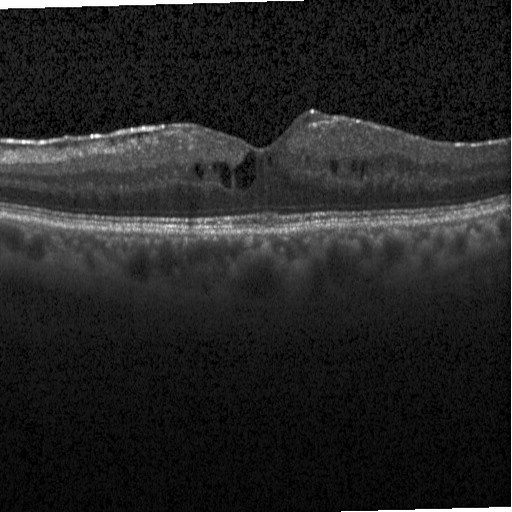

Finding: diabetic macular edema (DME).